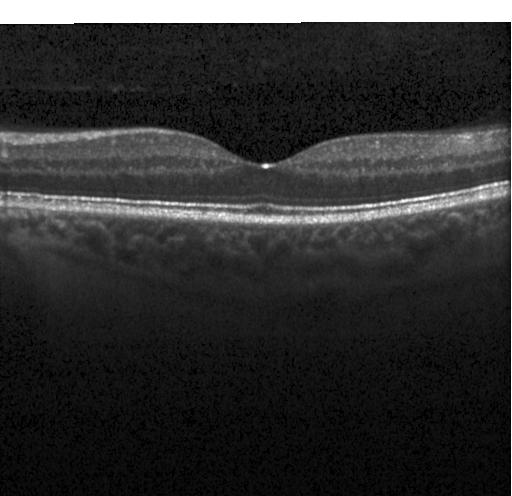
SD-OCT. Retinal OCT B-scan — Dx: no choroidal neovascularization, diabetic macular edema, or drusen.